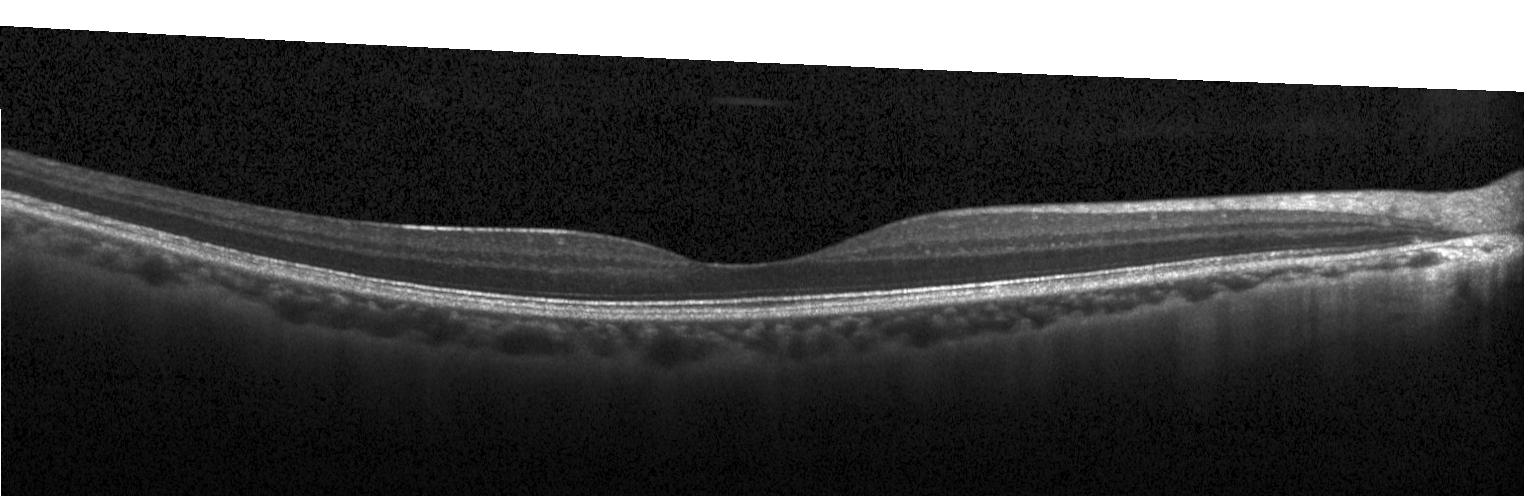

Spectral-domain OCT B-scan: no evidence of choroidal neovascularization, diabetic macular edema, or drusen.